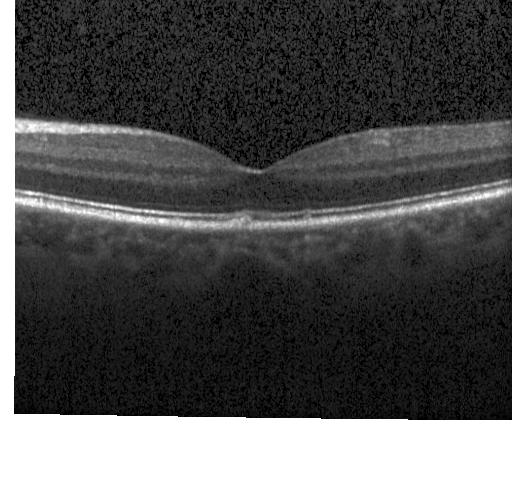
Macular OCT demonstrating sub-RPE drusenoid deposits.